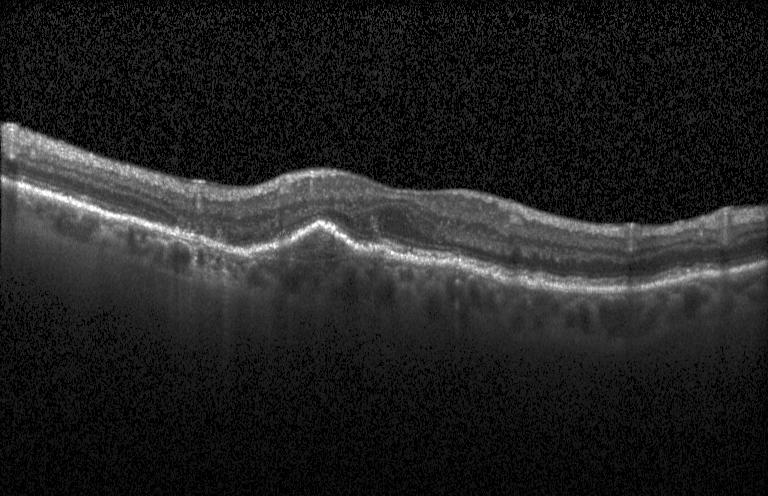 Impression: choroidal neovascularization (CNV).